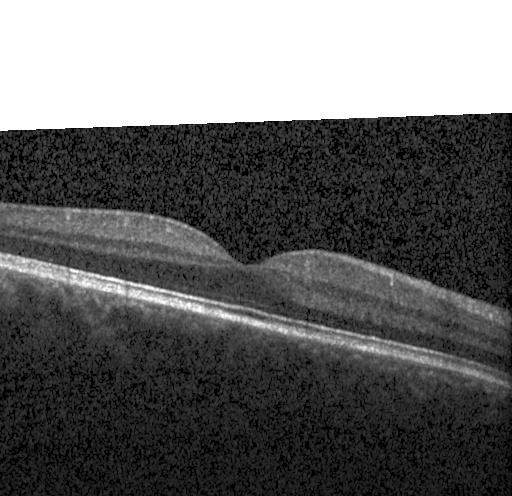

Optical coherence tomography scan. Spectral-domain optical coherence tomography. Heidelberg Spectralis. Fovea-centered.
The scan shows no evidence of CNV, DME, or drusen.